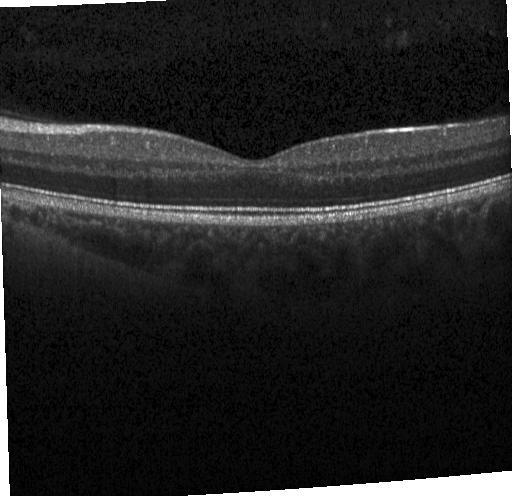 OCT finding: no evidence of choroidal neovascularization, diabetic macular edema, or drusen.